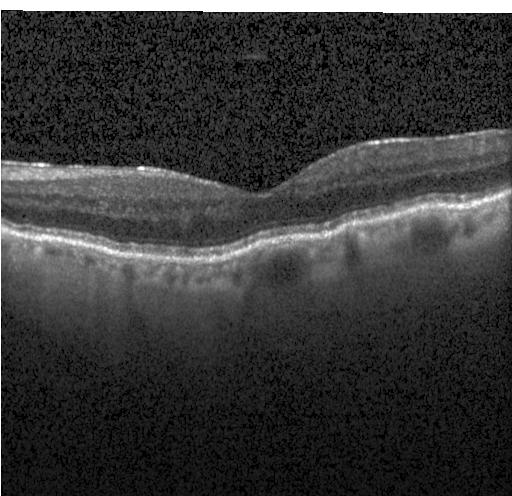 OCT B-scan · spectral-domain optical coherence tomography · macular scan · acquired on a Heidelberg Spectralis.
The scan shows no evidence of choroidal neovascularization, diabetic macular edema, or drusen.